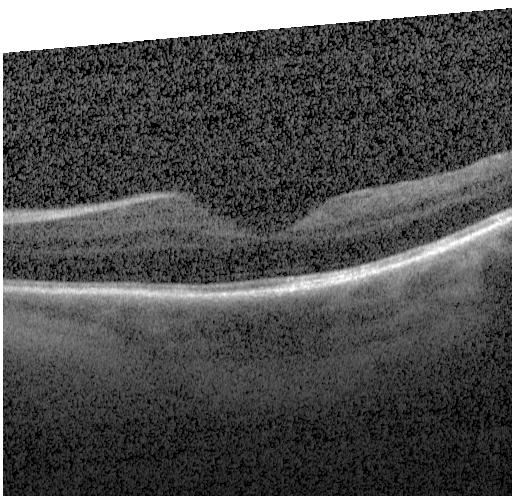

Retinal OCT B-scan.
No CNV, DME, or drusen.